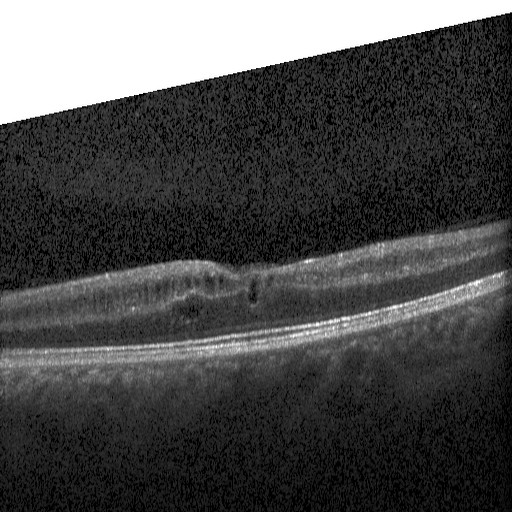
Acquired on a Heidelberg Spectralis · fovea-centered · spectral-domain OCT · optical coherence tomography scan — This B-scan demonstrates diabetic macular edema (DME).